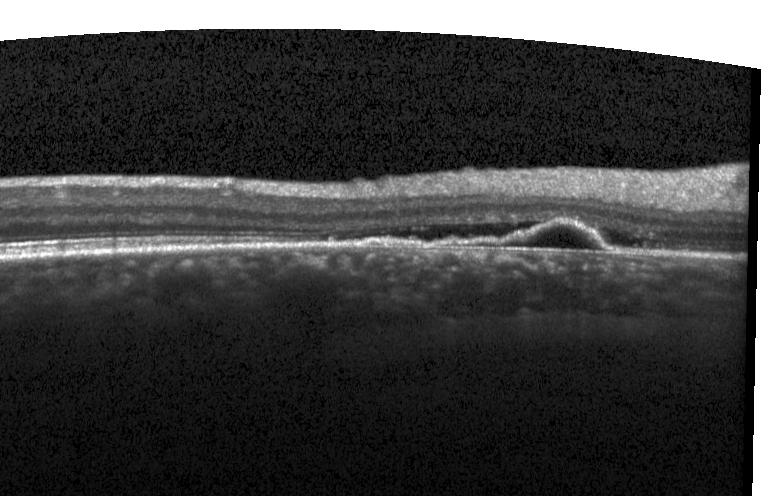 Optical coherence tomography B-scan
Diagnosis: choroidal neovascularization (CNV).